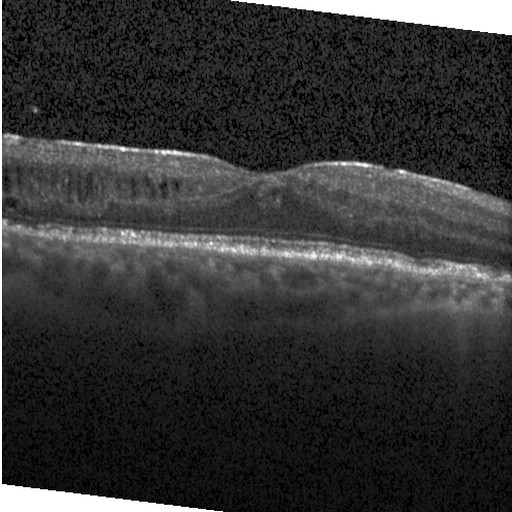
OCT line scan · SD-OCT · horizontal scan through the fovea · Heidelberg Spectralis — OCT finding: diabetic macular edema (DME).